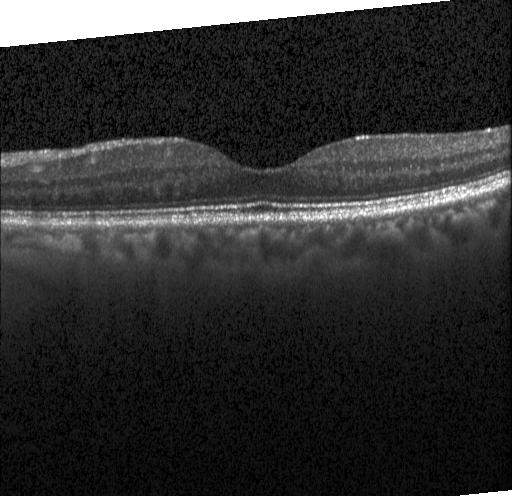

Horizontal scan through the fovea. OCT B-scan.
Assessment: no evidence of CNV, DME, or drusen.